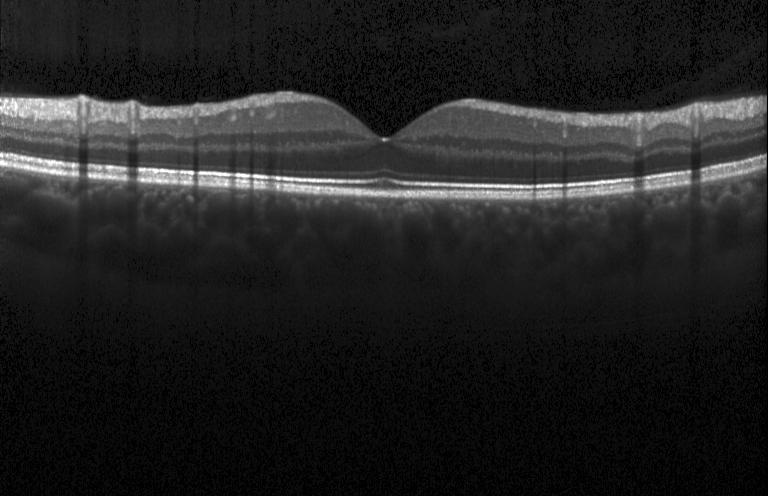 Centered on the fovea. Instrument: Heidelberg Spectralis. Retinal OCT B-scan. The scan shows no choroidal neovascularization, no diabetic macular edema, and no drusen.